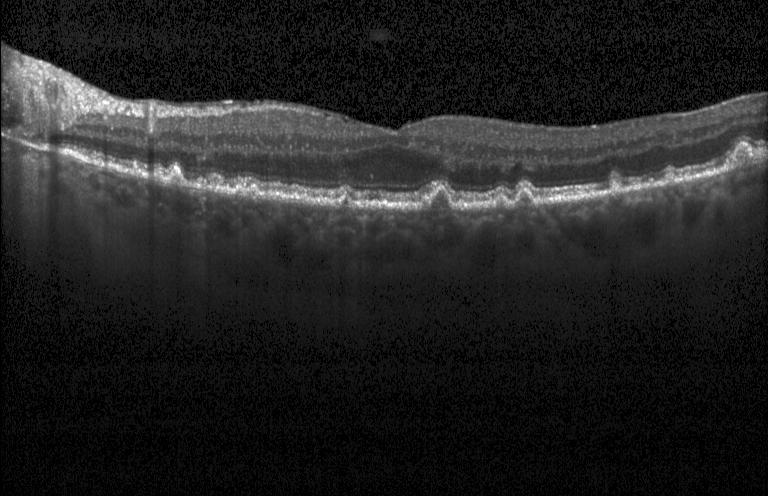
Fovea-centered, spectral-domain OCT, retinal OCT cross-section — Macular OCT: drusen.